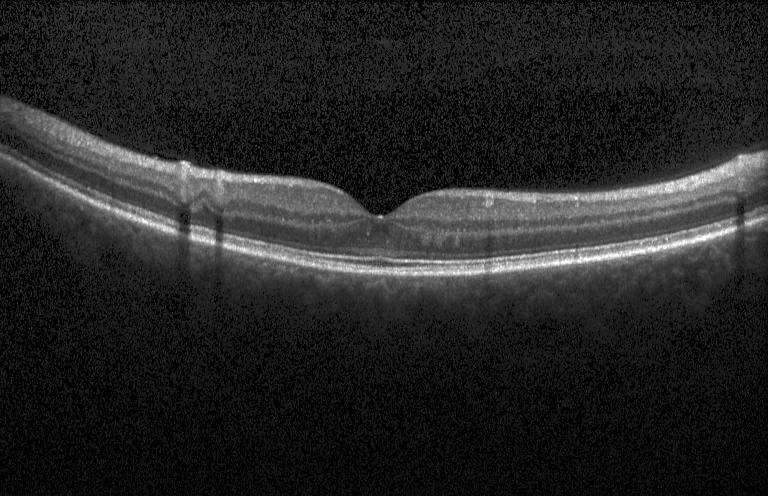 SD-OCT, retinal OCT cross-section.
Macular OCT: no choroidal neovascularization, no diabetic macular edema, and no drusen.